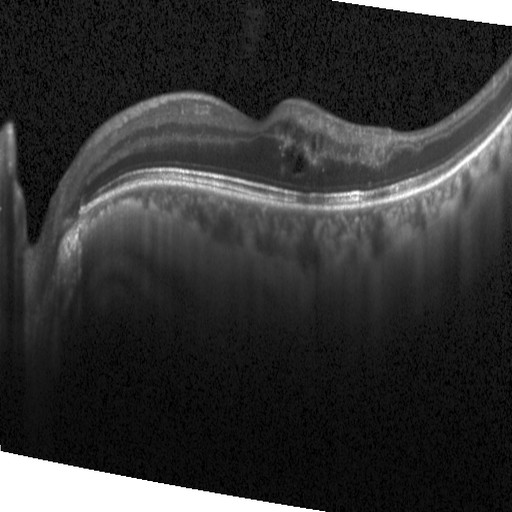
Spectral-domain OCT · centered on the fovea · OCT line scan · instrument: Heidelberg Spectralis — Diabetic macular edema.